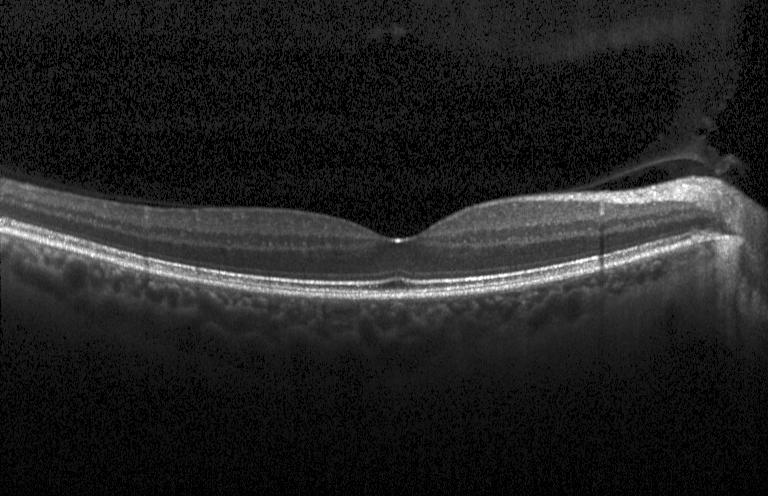

Dx: neither choroidal neovascularization, diabetic macular edema, nor drusen.